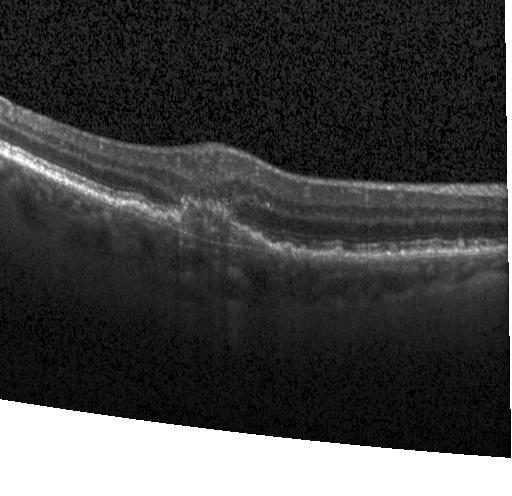

OCT line scan · centered on the fovea
Impression: a choroidal neovascular membrane.